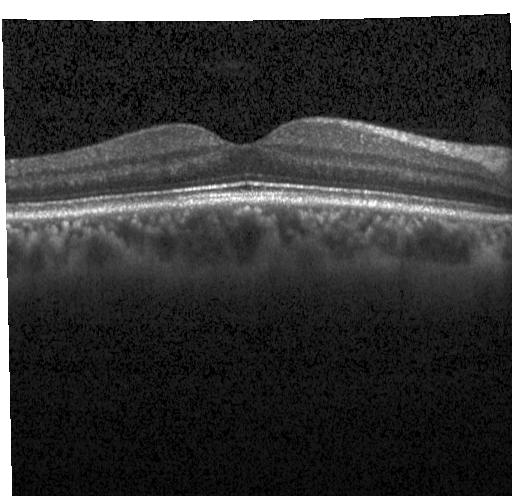

Spectral-domain OCT; macular scan; OCT line scan — Diagnosis: no choroidal neovascularization, diabetic macular edema, or drusen.